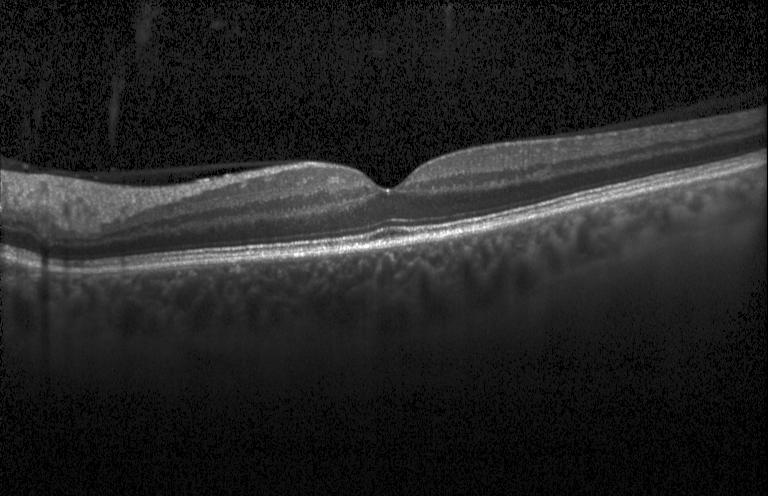 OCT B-scan showing no CNV, no DME, and no drusen.